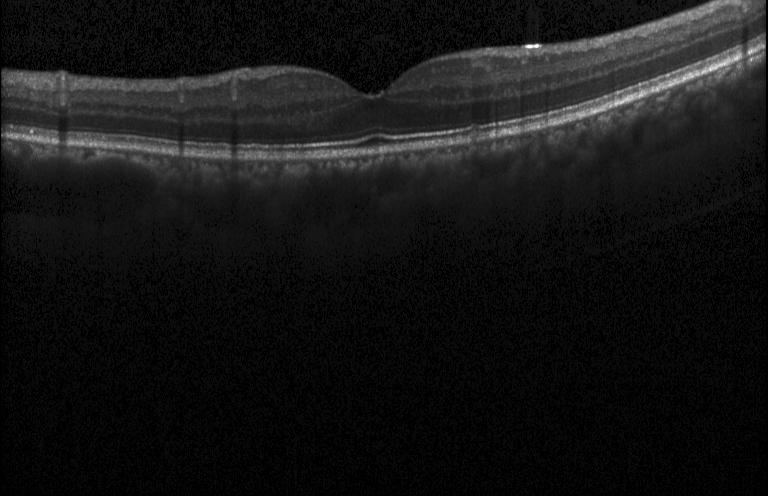

Impression: neither choroidal neovascularization, diabetic macular edema, nor drusen.